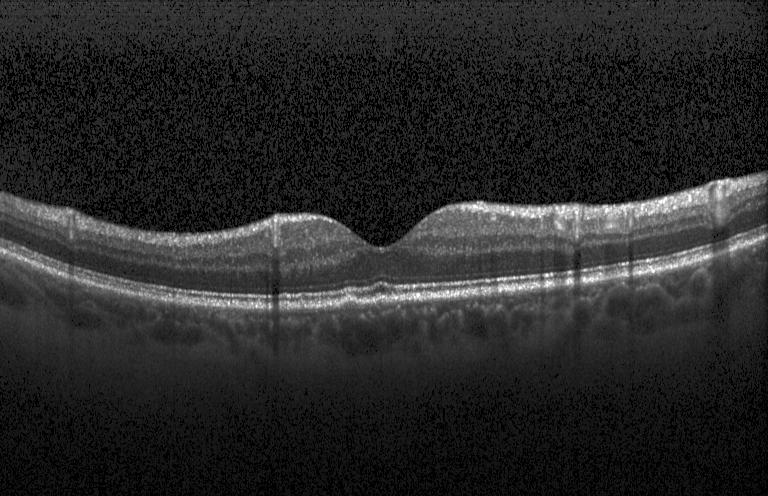
Spectral-domain OCT, retinal OCT B-scan. Finding: multiple drusen.